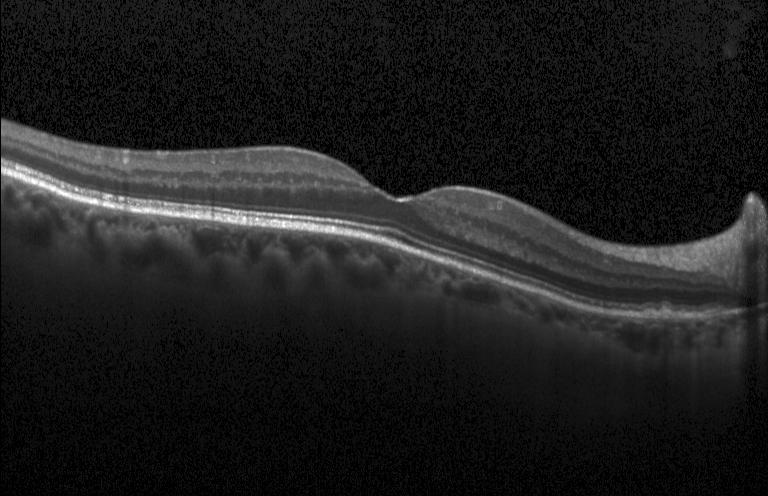

This B-scan demonstrates no CNV, DME, or drusen.